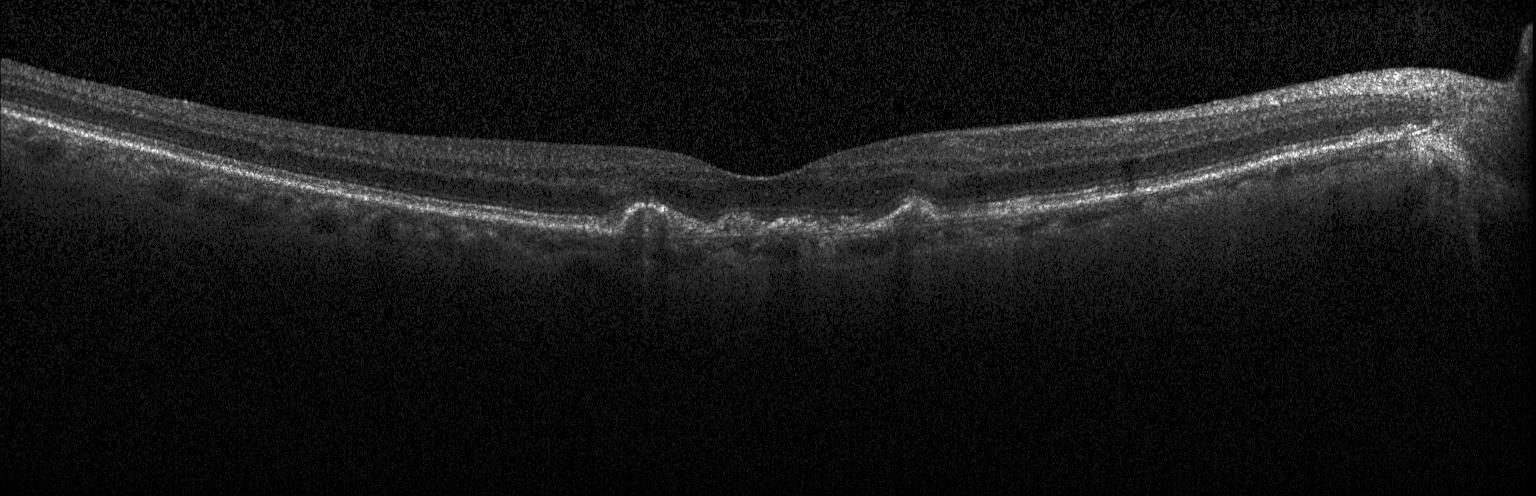 Retinal OCT cross-section showing multiple drusen.